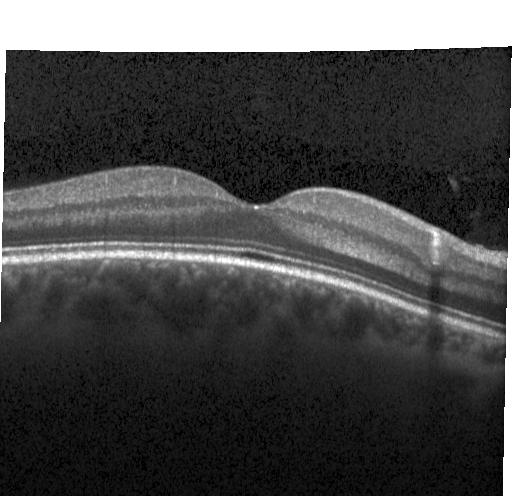

Acquired on a Heidelberg Spectralis · OCT line scan · macular scan · spectral-domain optical coherence tomography. Macular OCT: no choroidal neovascularization, diabetic macular edema, or drusen.